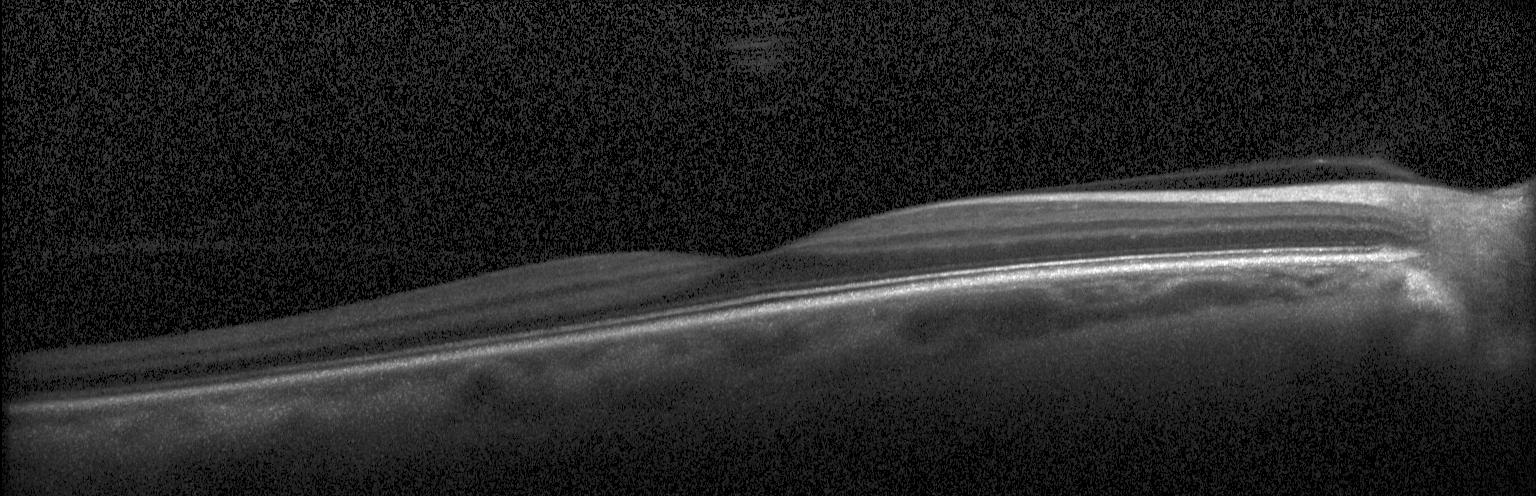 Optical coherence tomography scan. Finding: no choroidal neovascularization, no diabetic macular edema, and no drusen.